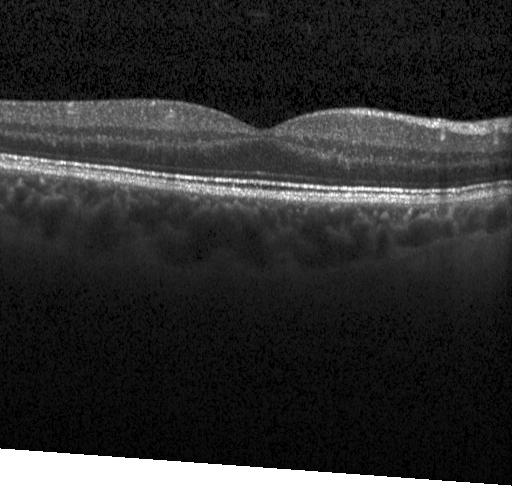
Optical coherence tomography scan
Impression: no choroidal neovascularization, diabetic macular edema, or drusen.